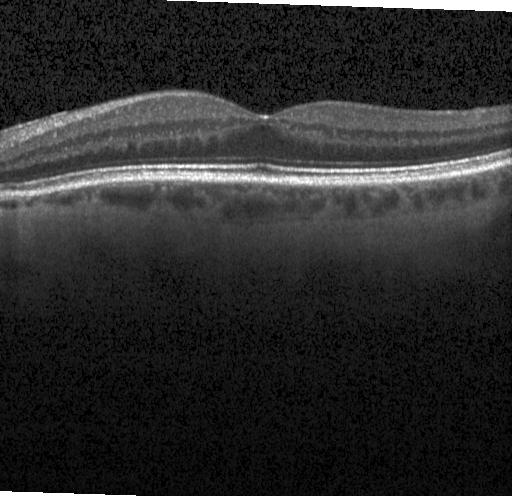
Retinal OCT cross-section, Heidelberg Spectralis, macular scan. Impression: neither choroidal neovascularization, diabetic macular edema, nor drusen.